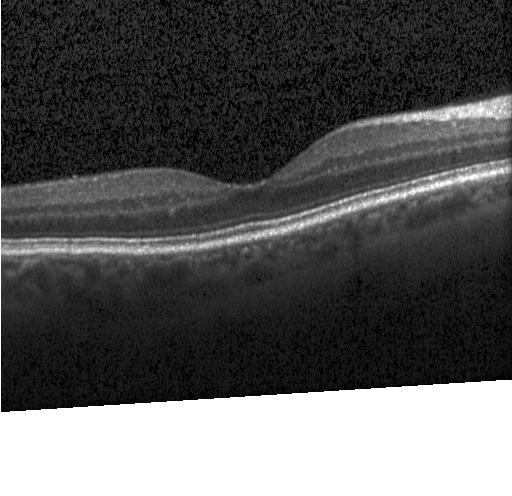
Finding: neither choroidal neovascularization, diabetic macular edema, nor drusen.